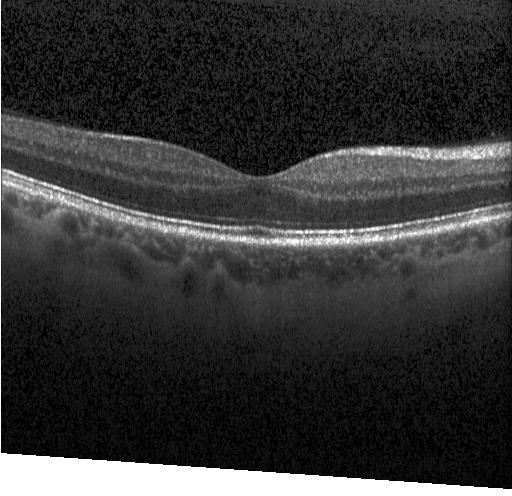
Optical coherence tomography B-scan, fovea-centered, SD-OCT, acquired on a Heidelberg Spectralis
Diagnosis: neither choroidal neovascularization, diabetic macular edema, nor drusen.